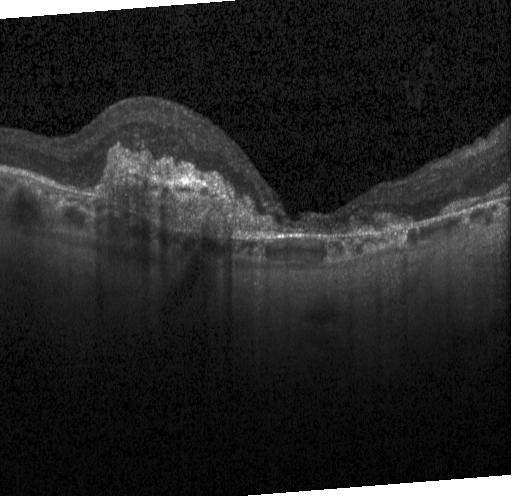 Spectral-domain optical coherence tomography, optical coherence tomography B-scan, acquired on a Heidelberg Spectralis, macular scan. The scan shows a choroidal neovascular membrane.